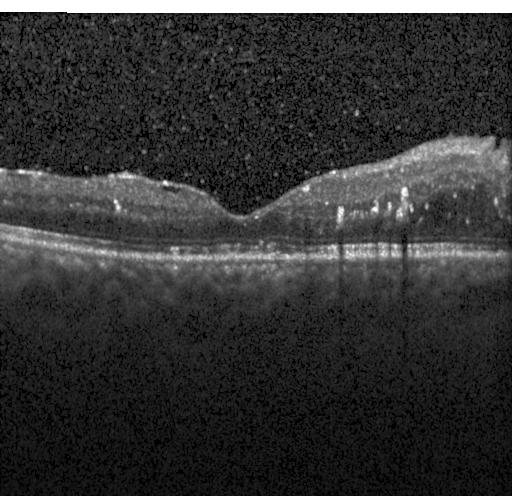
Horizontal scan through the fovea. OCT line scan. SD-OCT. Heidelberg Spectralis — Diagnosis: DME.